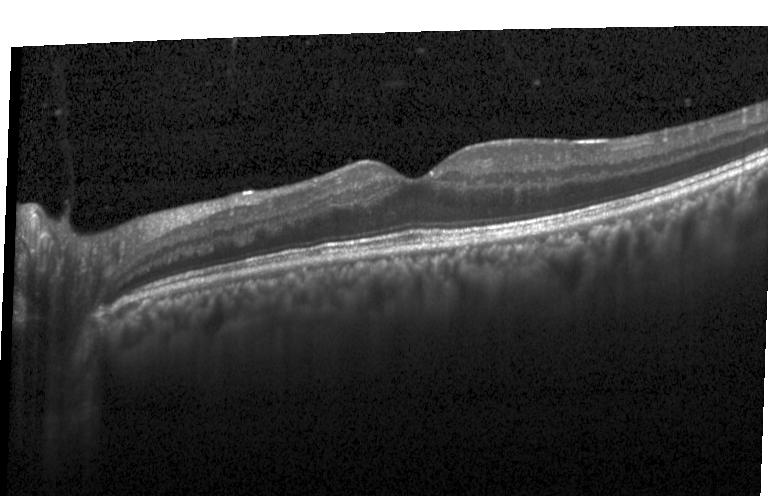

Retinal OCT cross-section · spectral-domain optical coherence tomography — No choroidal neovascularization, no diabetic macular edema, and no drusen.